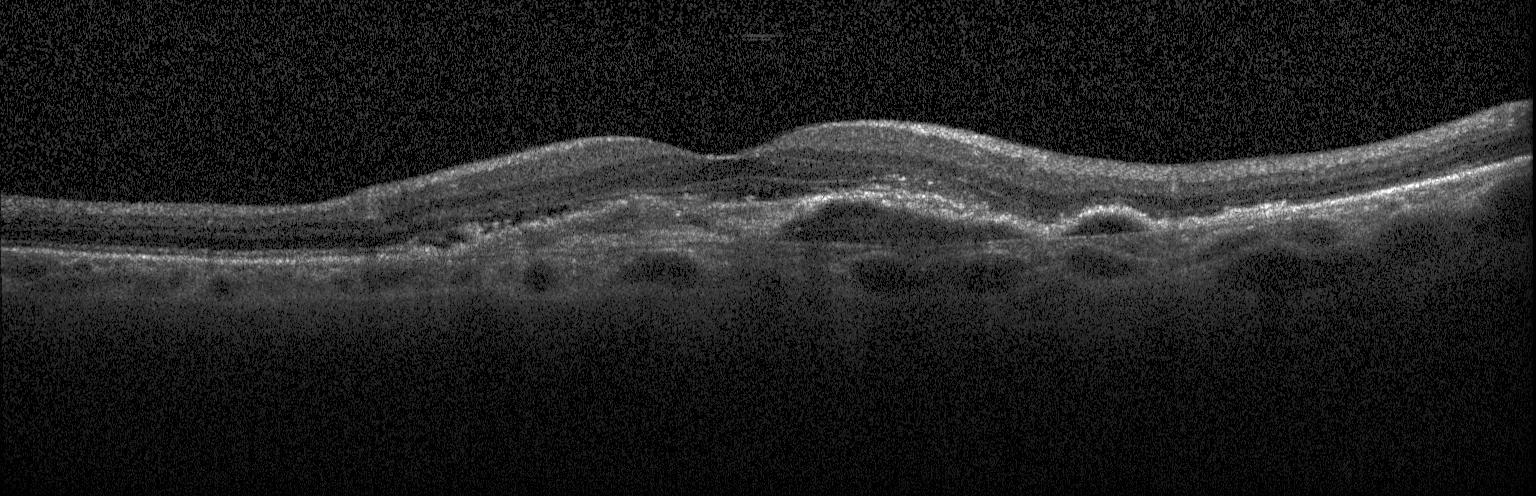
OCT line scan · fovea-centered · spectral-domain OCT — Impression: a choroidal neovascular membrane.